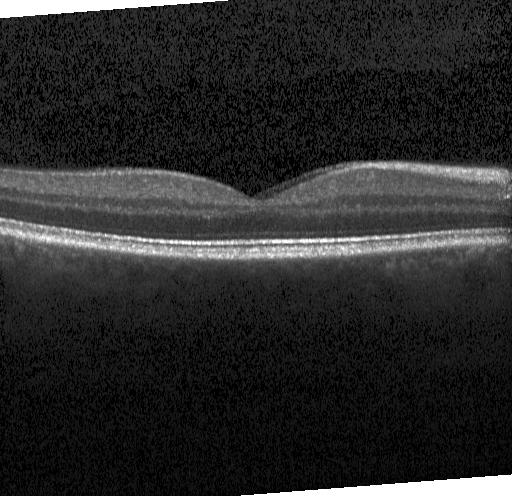

Spectral-domain optical coherence tomography; acquired on a Heidelberg Spectralis; macular scan; OCT line scan — Assessment: neither CNV, DME, nor drusen.